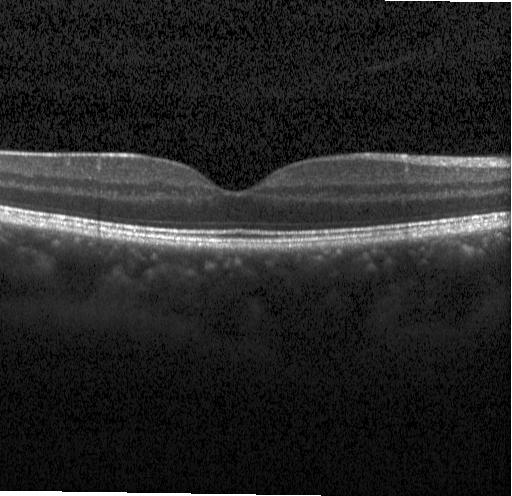

OCT scan showing neither CNV, DME, nor drusen.